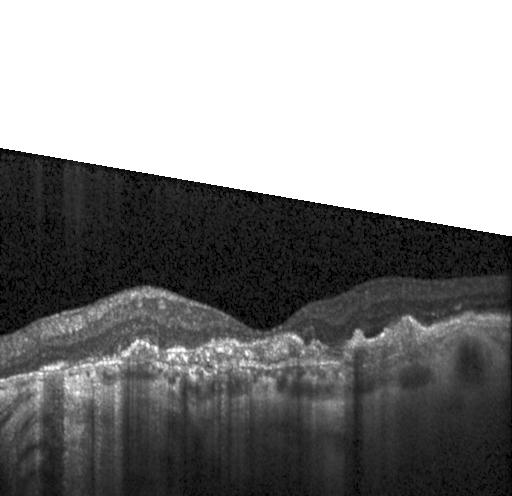

OCT line scan
Macular OCT: CNV.